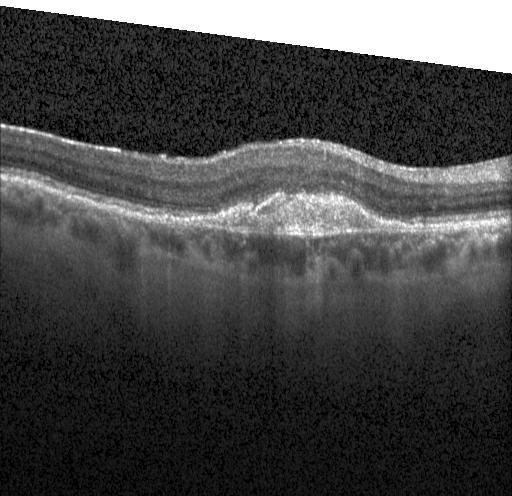

Horizontal scan through the fovea, optical coherence tomography scan
Finding: a choroidal neovascular membrane.